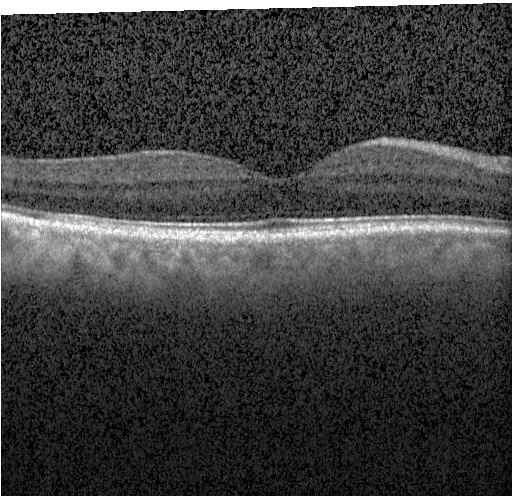 Retinal OCT cross-section; SD-OCT; Heidelberg Spectralis.
Assessment: no evidence of choroidal neovascularization, diabetic macular edema, or drusen.